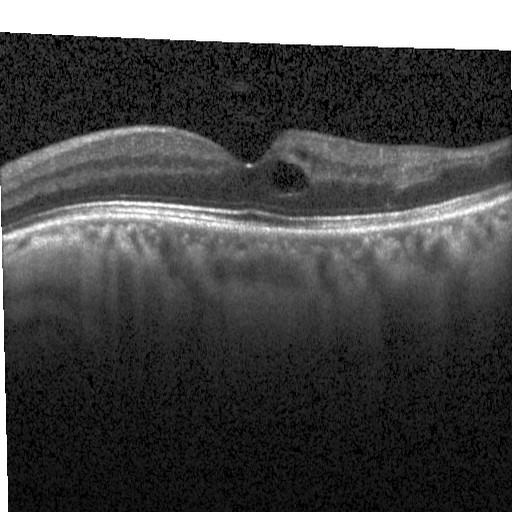

Optical coherence tomography B-scan, Heidelberg Spectralis. This B-scan demonstrates diabetic macular edema.